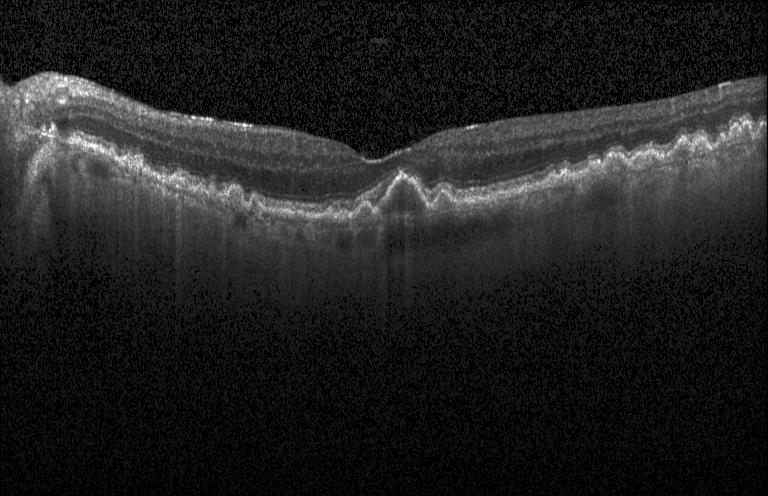 Retinal OCT B-scan, spectral-domain OCT — Impression: drusen.